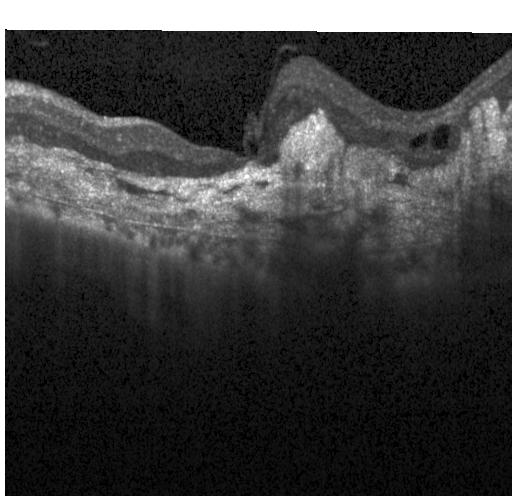
Fovea-centered; optical coherence tomography B-scan
The scan shows a choroidal neovascular membrane.